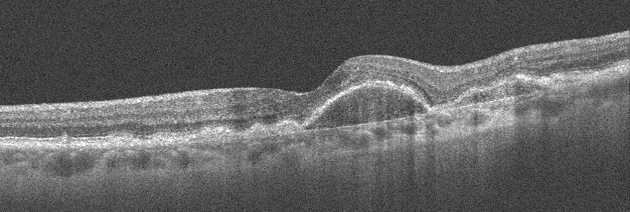
Optical coherence tomography B-scan · oculus sinister — Diagnosis: AMD.